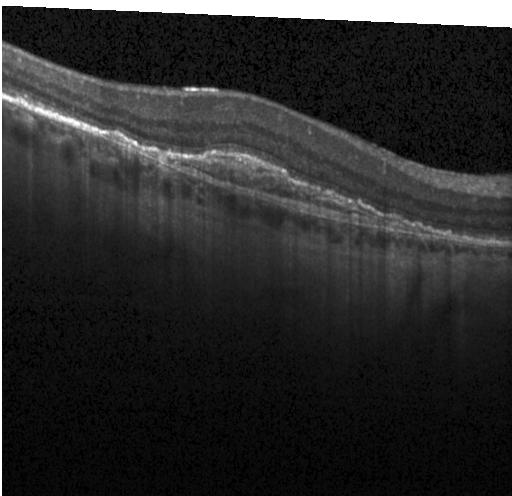

The scan shows choroidal neovascularization.